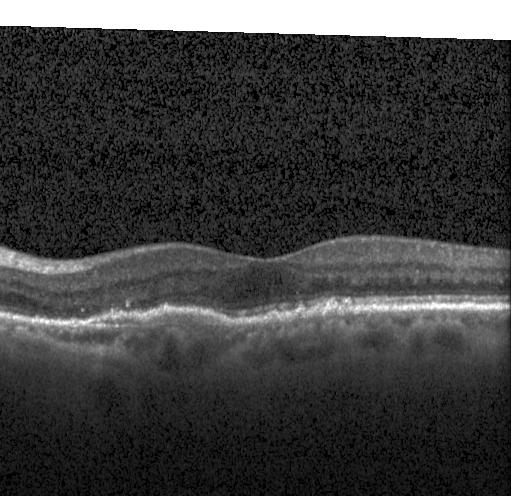

Acquired on a Heidelberg Spectralis; retinal OCT B-scan; centered on the fovea — Finding: a choroidal neovascular membrane.